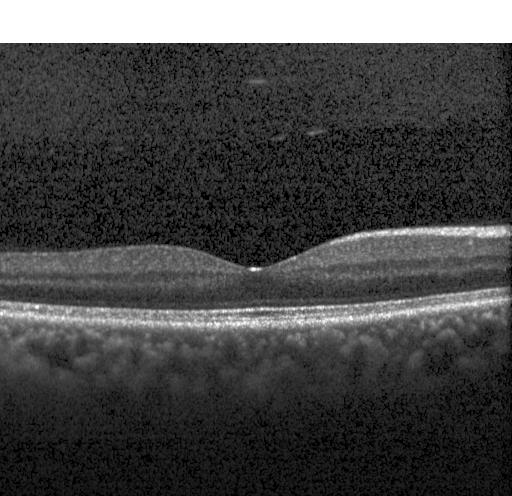 Optical coherence tomography B-scan
Diagnosis: no choroidal neovascularization, diabetic macular edema, or drusen.